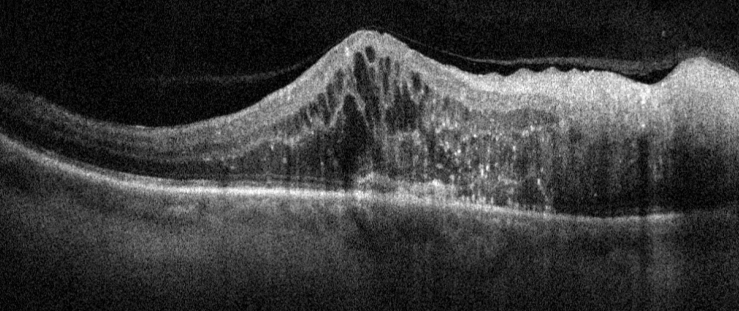

Impression: DME.